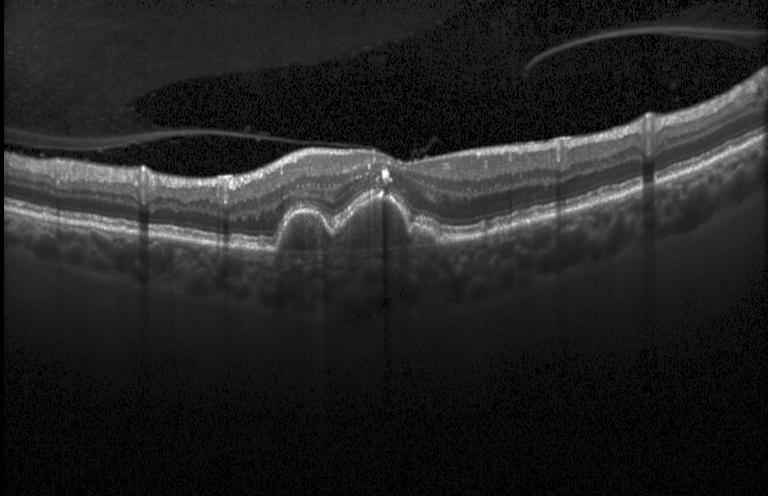

Spectral-domain OCT · Heidelberg Spectralis OCT system · OCT B-scan · horizontal scan through the fovea. Impression: a choroidal neovascular membrane.